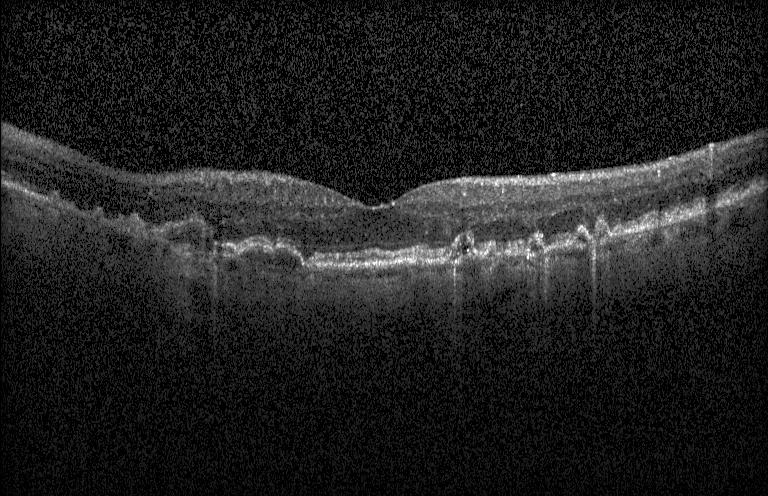

OCT B-scan showing a choroidal neovascular membrane.